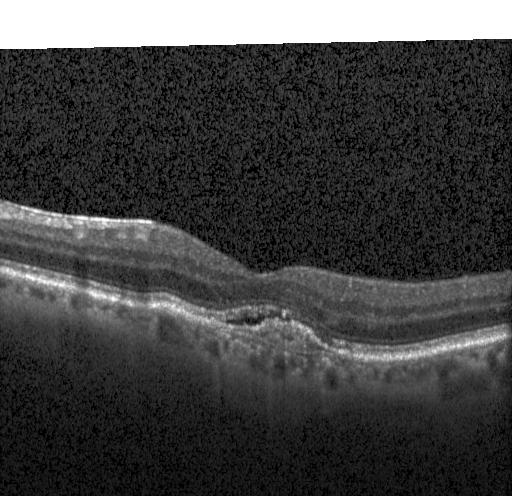 Diagnosis: a choroidal neovascular membrane.